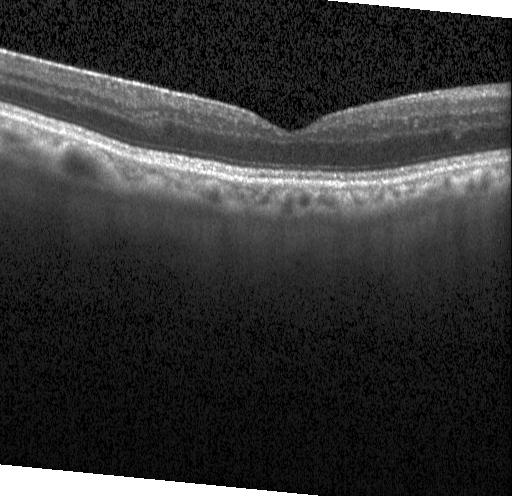
Retinal OCT B-scan.
Diagnosis: neither choroidal neovascularization, diabetic macular edema, nor drusen.